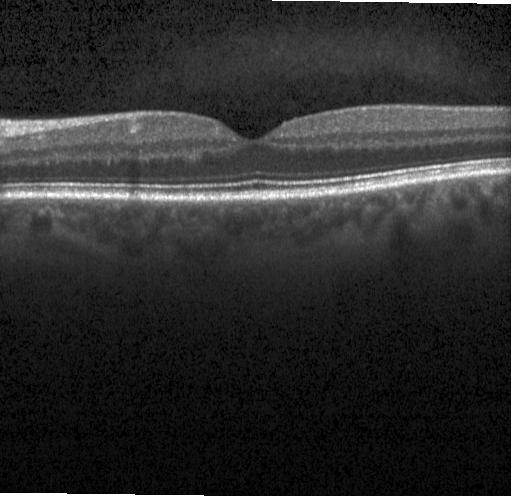 Retinal OCT cross-section
This B-scan demonstrates no CNV, no DME, and no drusen.